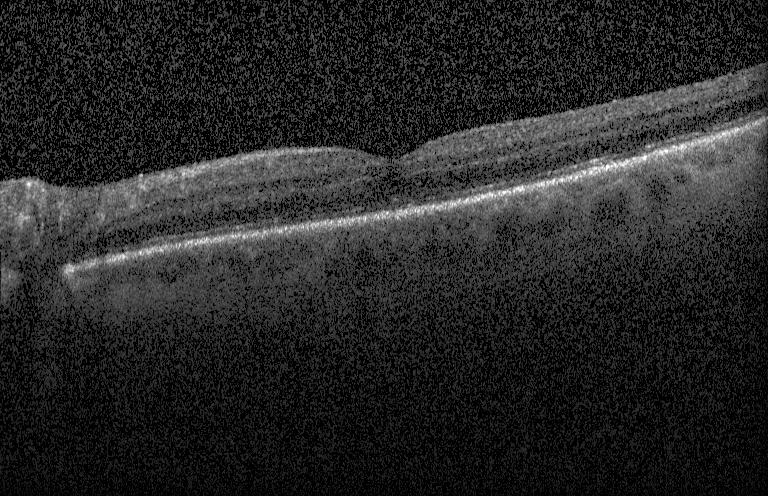
OCT B-scan. Finding: neither choroidal neovascularization, diabetic macular edema, nor drusen.